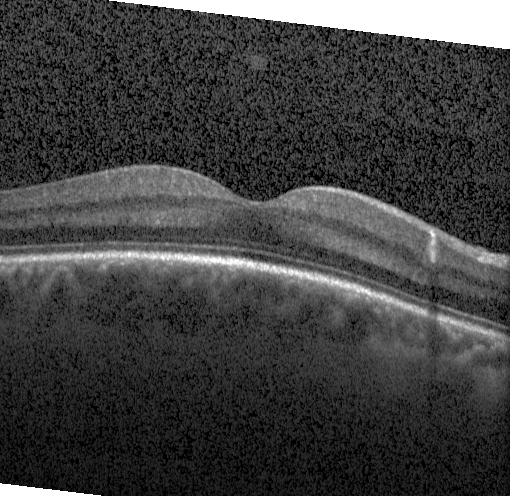
OCT line scan — Finding: neither choroidal neovascularization, diabetic macular edema, nor drusen.